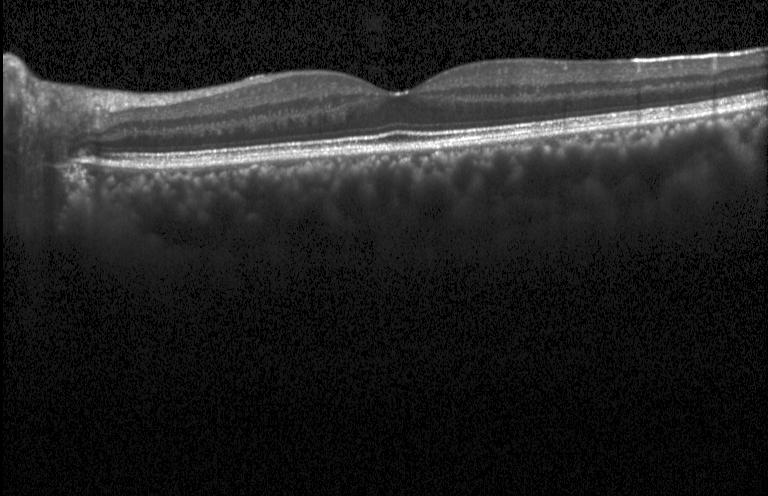 Spectral-domain OCT · OCT line scan · through the macula · instrument: Heidelberg Spectralis — Finding: neither choroidal neovascularization, diabetic macular edema, nor drusen.